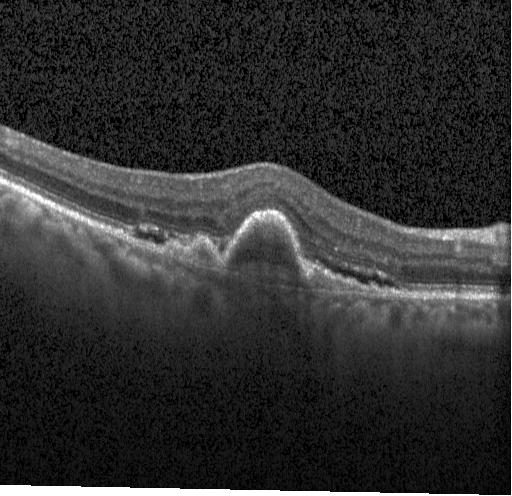 Finding: CNV.